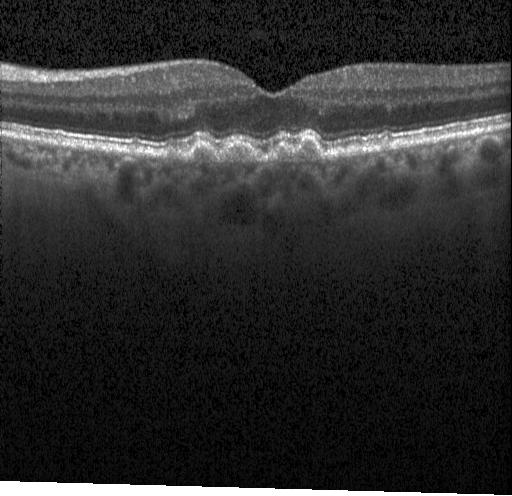 OCT line scan. Spectral-domain optical coherence tomography. Instrument: Heidelberg Spectralis — Diagnosis: sub-RPE drusenoid deposits.